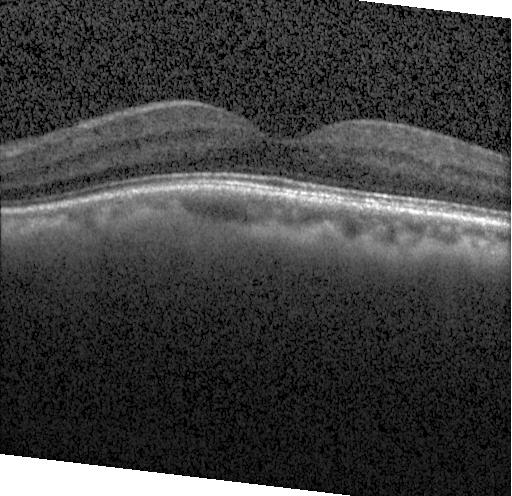
OCT scan showing neither choroidal neovascularization, diabetic macular edema, nor drusen.